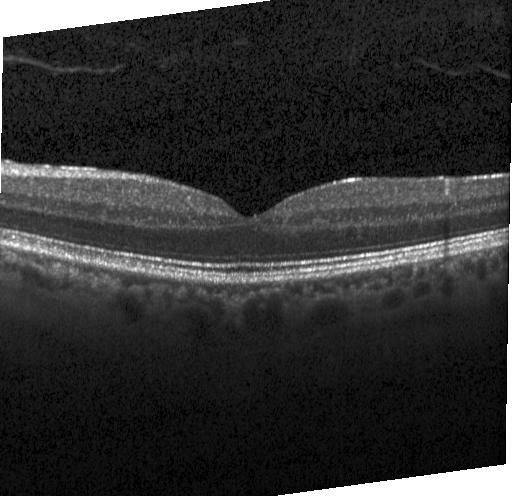
The scan shows no CNV, DME, or drusen.